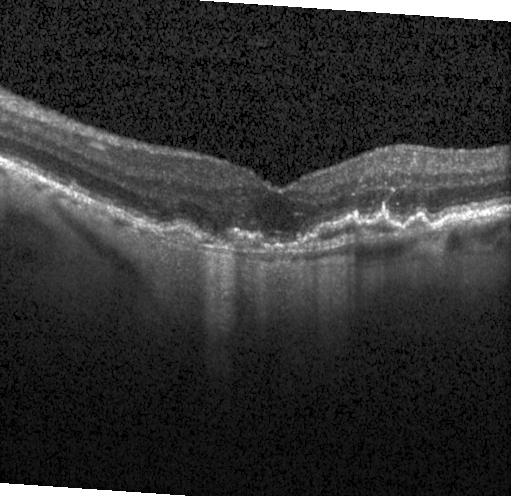 OCT line scan, horizontal scan through the fovea, SD-OCT — Finding: CNV.